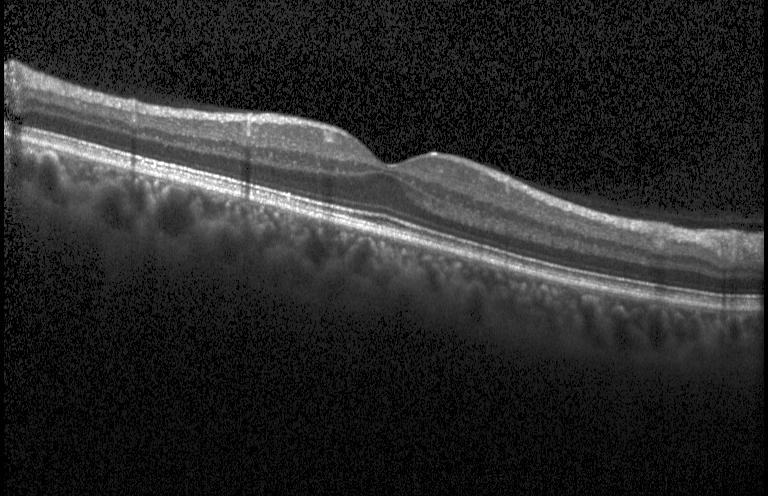

The scan shows no CNV, no DME, and no drusen.